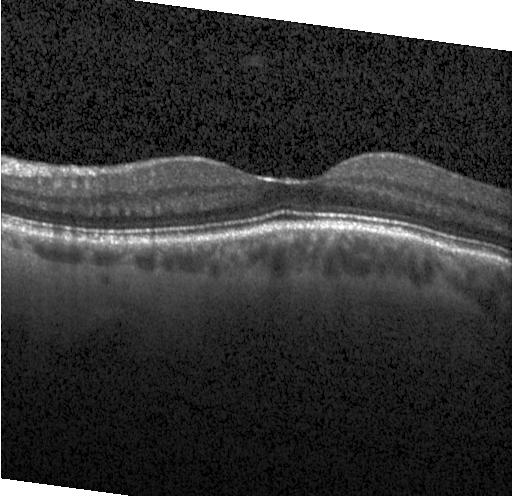

Retinal OCT cross-section. Macular OCT: no choroidal neovascularization, diabetic macular edema, or drusen.